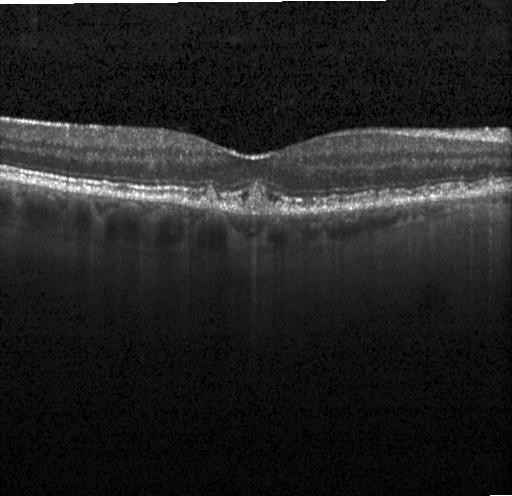 Optical coherence tomography B-scan
Finding: multiple drusen.